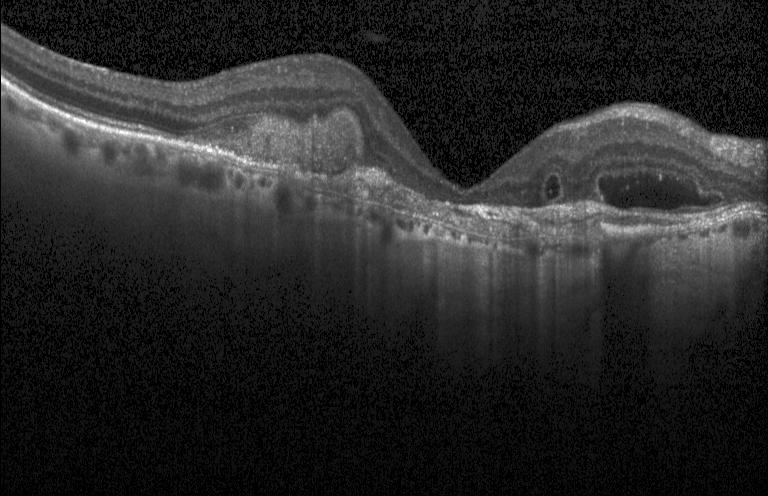

Dx: a choroidal neovascular membrane.